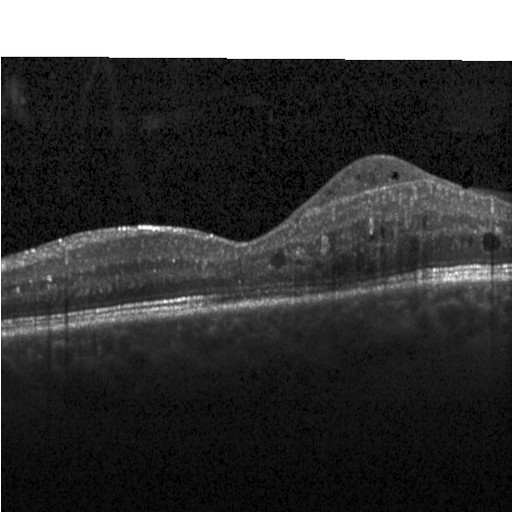 Fovea-centered; OCT B-scan; spectral-domain optical coherence tomography; acquired on a Heidelberg Spectralis.
This B-scan demonstrates diabetic macular edema (DME).